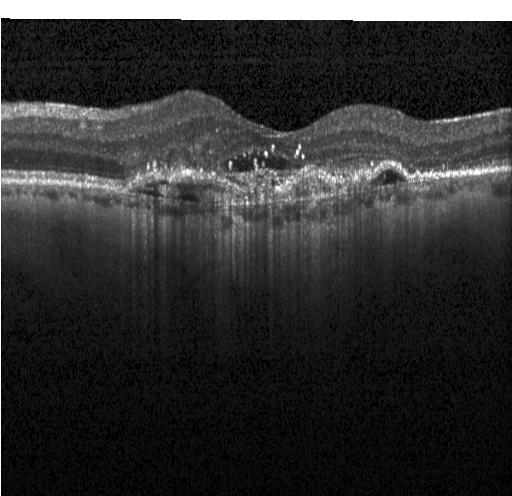 OCT finding: a choroidal neovascular membrane.